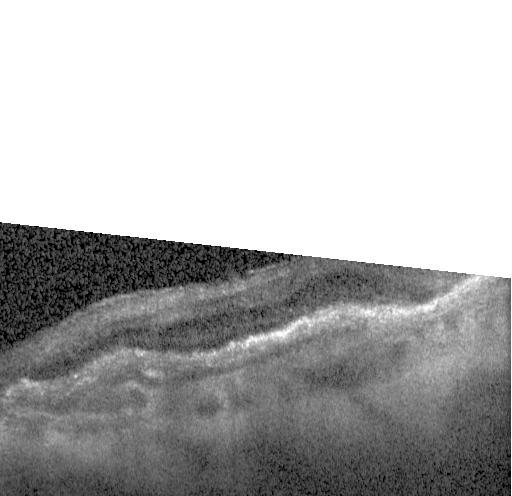

Retinal OCT cross-section; horizontal scan through the fovea
Assessment: CNV.